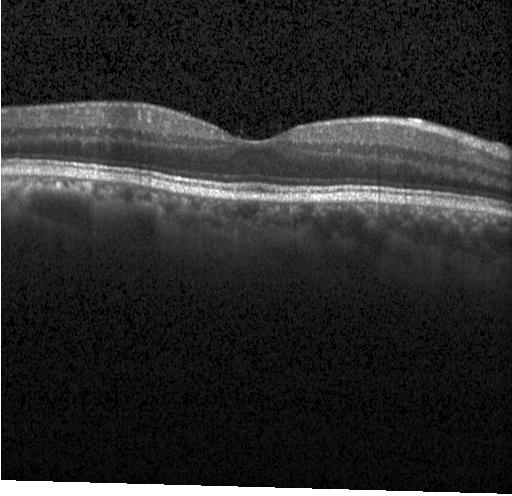 Spectral-domain optical coherence tomography · retinal OCT B-scan. This B-scan demonstrates no evidence of choroidal neovascularization, diabetic macular edema, or drusen.